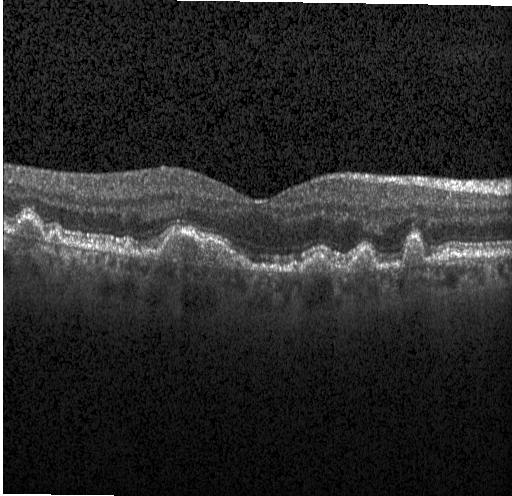 Heidelberg Spectralis OCT system, SD-OCT, optical coherence tomography scan.
The scan shows multiple drusen.